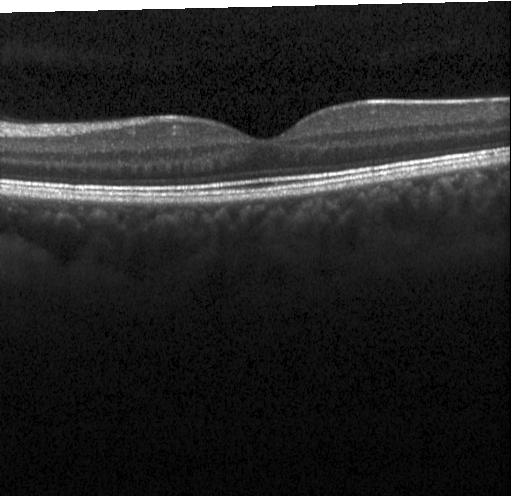 Finding: no evidence of CNV, DME, or drusen.